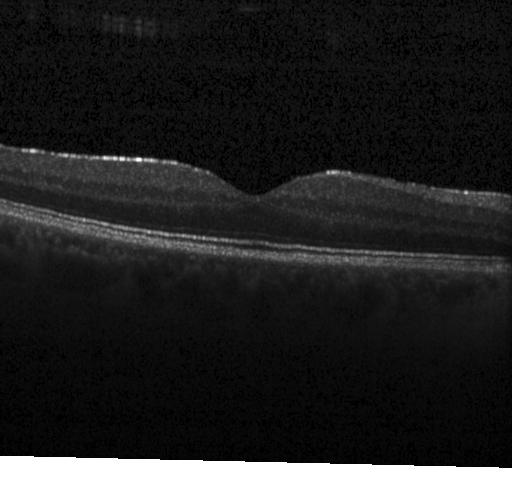
Retinal OCT cross-section; spectral-domain OCT; Heidelberg Spectralis OCT system — OCT finding: no evidence of choroidal neovascularization, diabetic macular edema, or drusen.